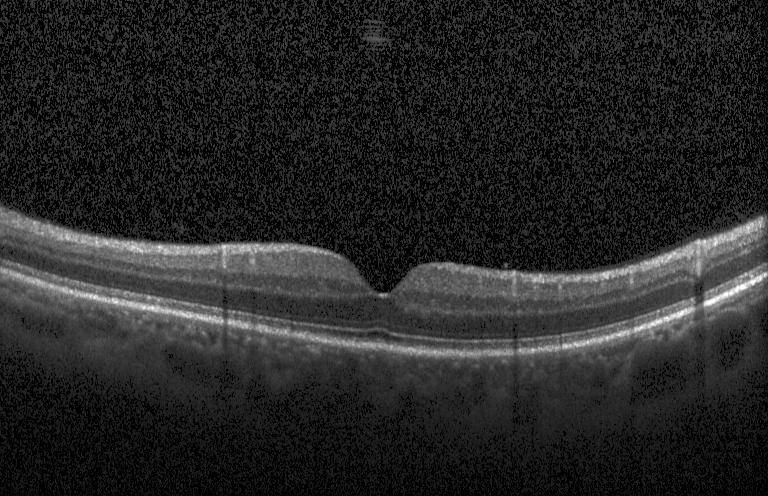 Optical coherence tomography scan; macular scan; spectral-domain optical coherence tomography; acquired on a Heidelberg Spectralis. Diagnosis: no CNV, no DME, and no drusen.